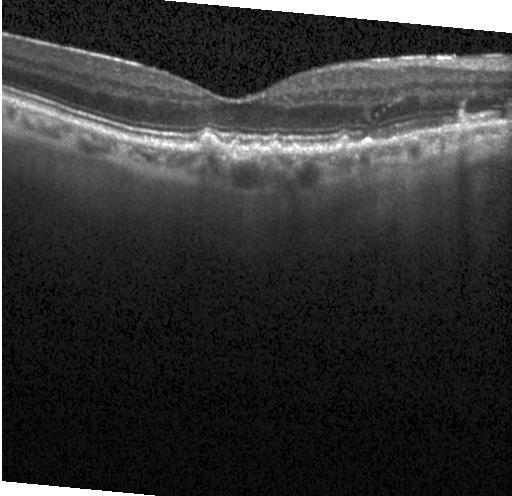

Finding: multiple drusen.